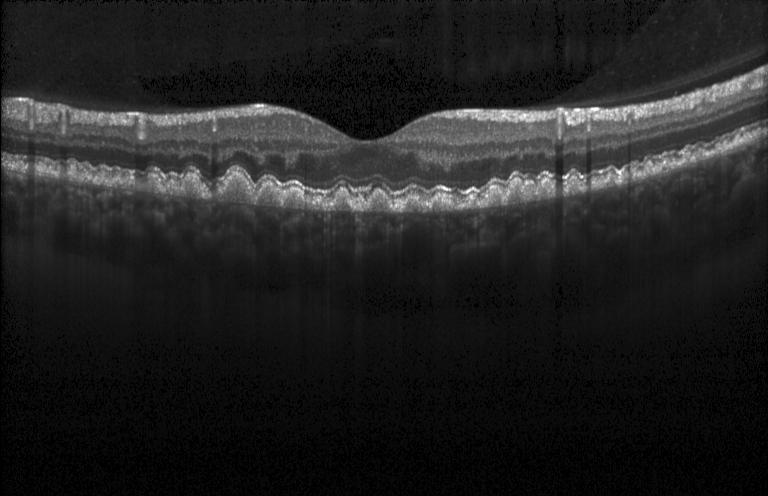 Retinal OCT cross-section showing sub-RPE drusenoid deposits.